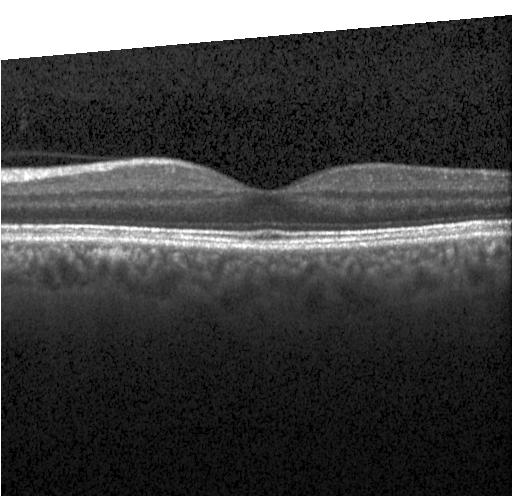
OCT line scan. Spectral-domain optical coherence tomography. Horizontal scan through the fovea — This B-scan demonstrates no choroidal neovascularization, diabetic macular edema, or drusen.